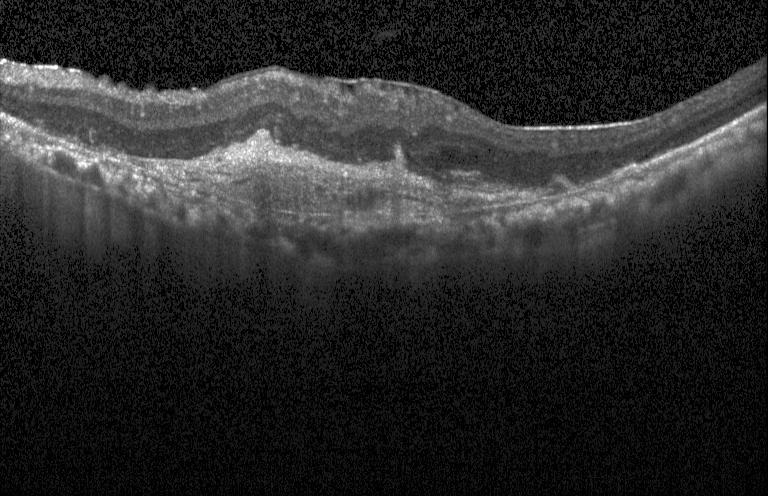

Retinal OCT B-scan · spectral-domain optical coherence tomography.
Finding: a choroidal neovascular membrane.